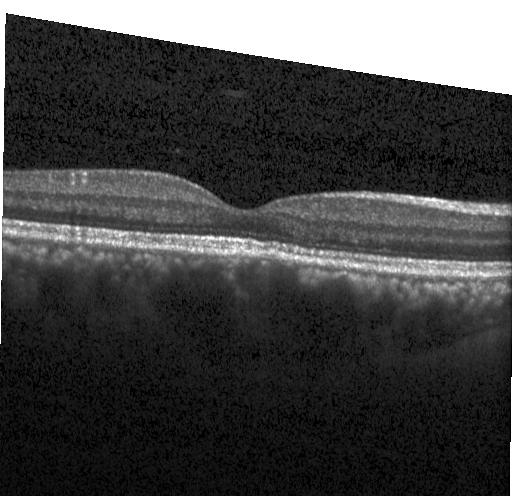
Heidelberg Spectralis OCT system · spectral-domain OCT · horizontal scan through the fovea · OCT B-scan
Impression: no evidence of choroidal neovascularization, diabetic macular edema, or drusen.